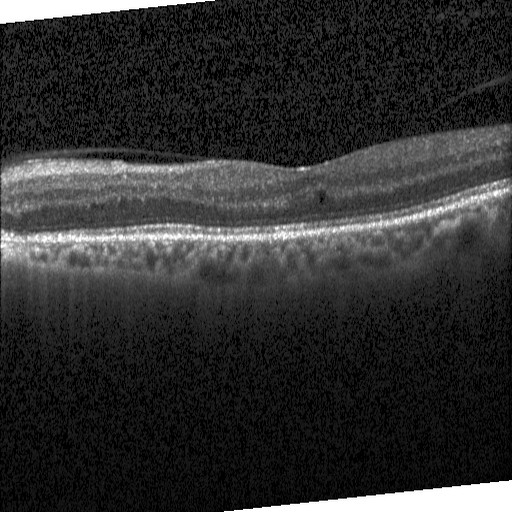 Optical coherence tomography scan · horizontal scan through the fovea. Diagnosis: diabetic macular edema (DME).